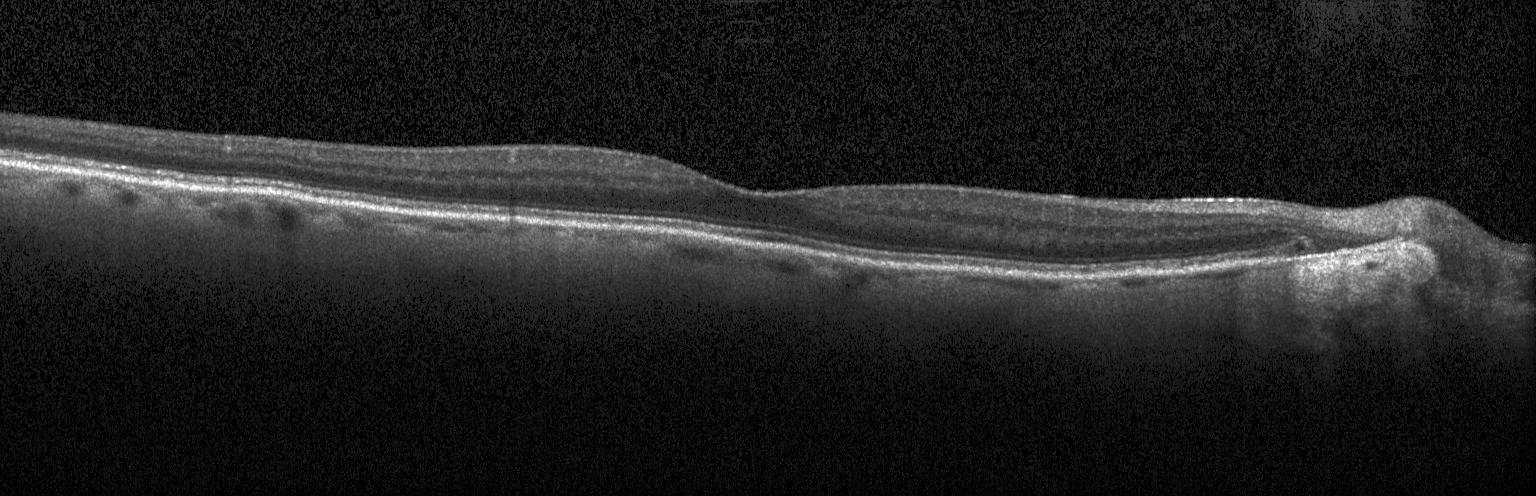

The scan shows no CNV, DME, or drusen.